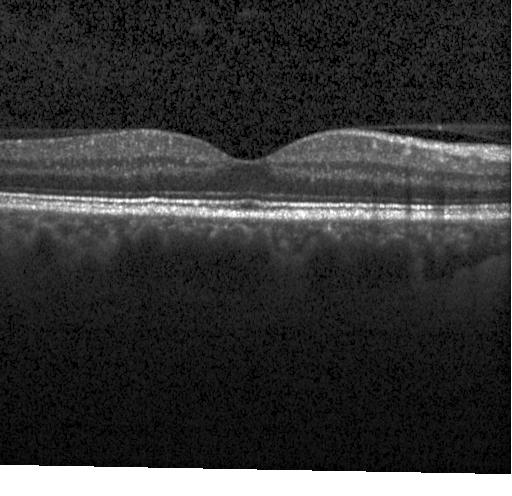
Spectral-domain OCT B-scan: no choroidal neovascularization, diabetic macular edema, or drusen.